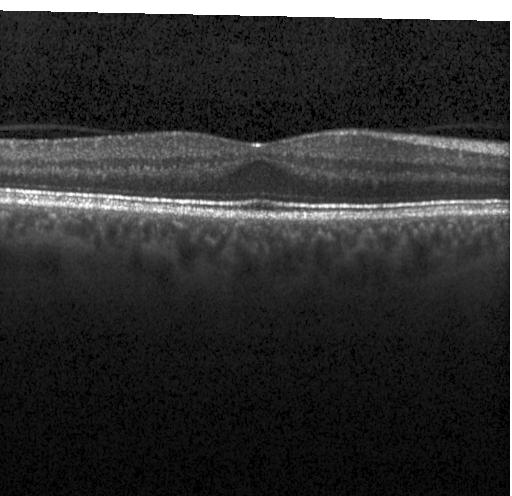

Horizontal scan through the fovea. OCT B-scan — Finding: neither CNV, DME, nor drusen.